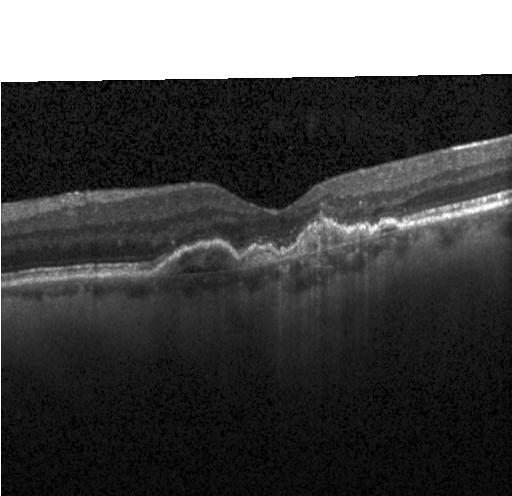 OCT B-scan showing a choroidal neovascular membrane.